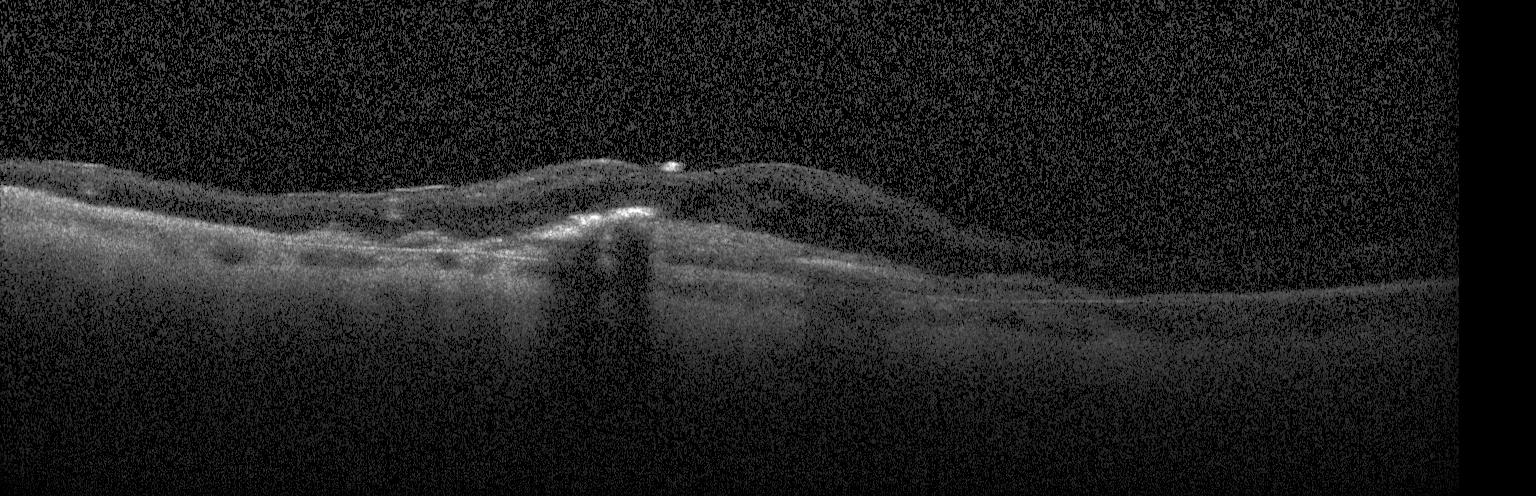 Macular OCT: a choroidal neovascular membrane.